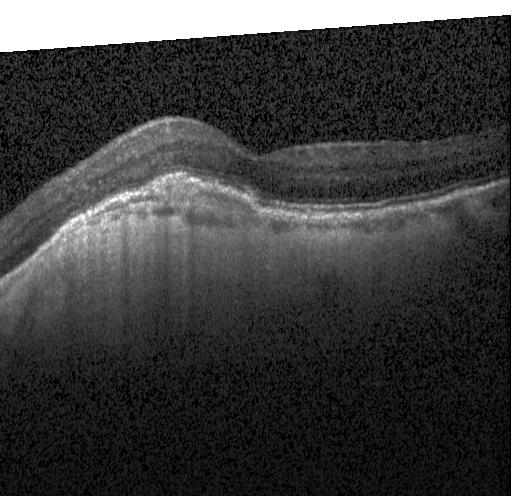

Finding: CNV.